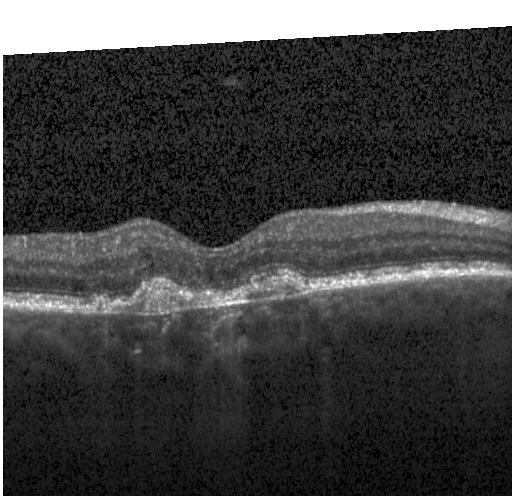
Choroidal neovascularization (CNV).